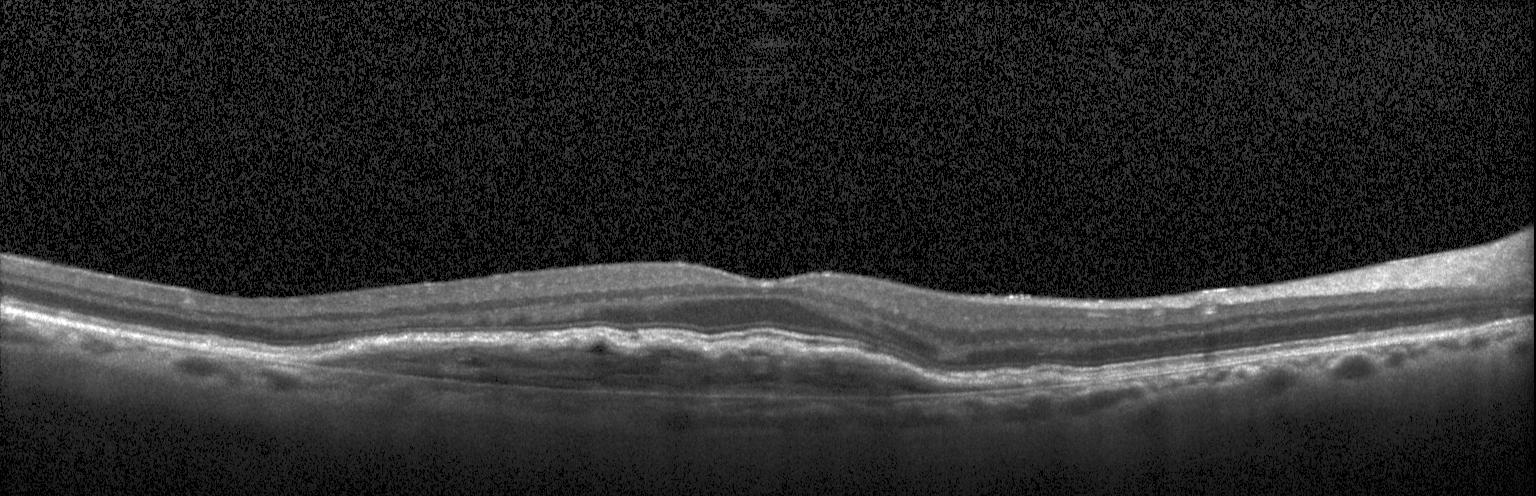

Acquired on a Heidelberg Spectralis. Optical coherence tomography B-scan. Centered on the fovea. SD-OCT.
Assessment: a choroidal neovascular membrane.